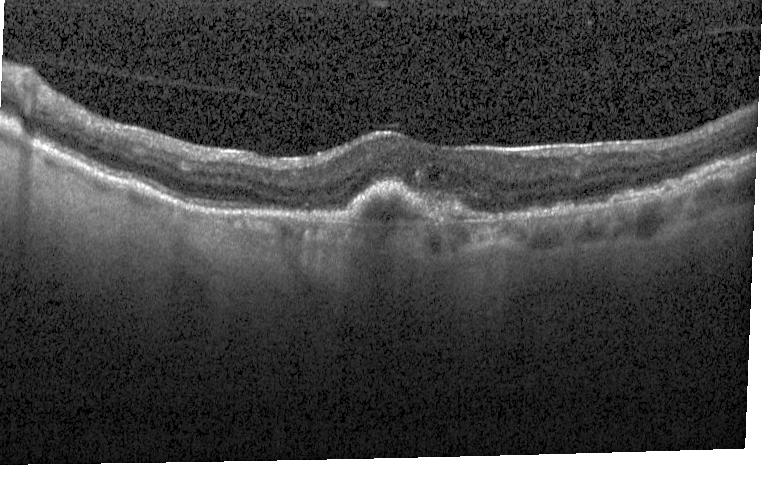 Retinal OCT B-scan. A choroidal neovascular membrane.